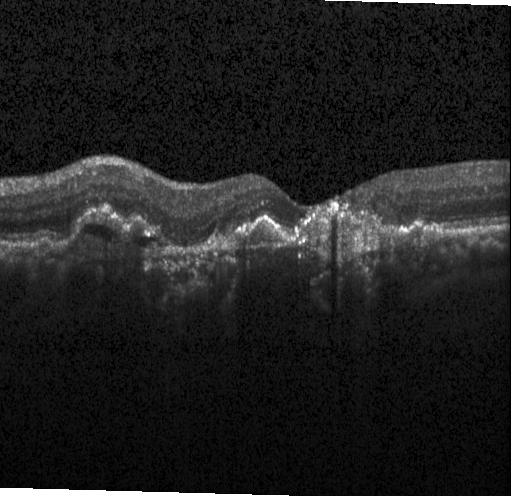 OCT line scan. CNV.